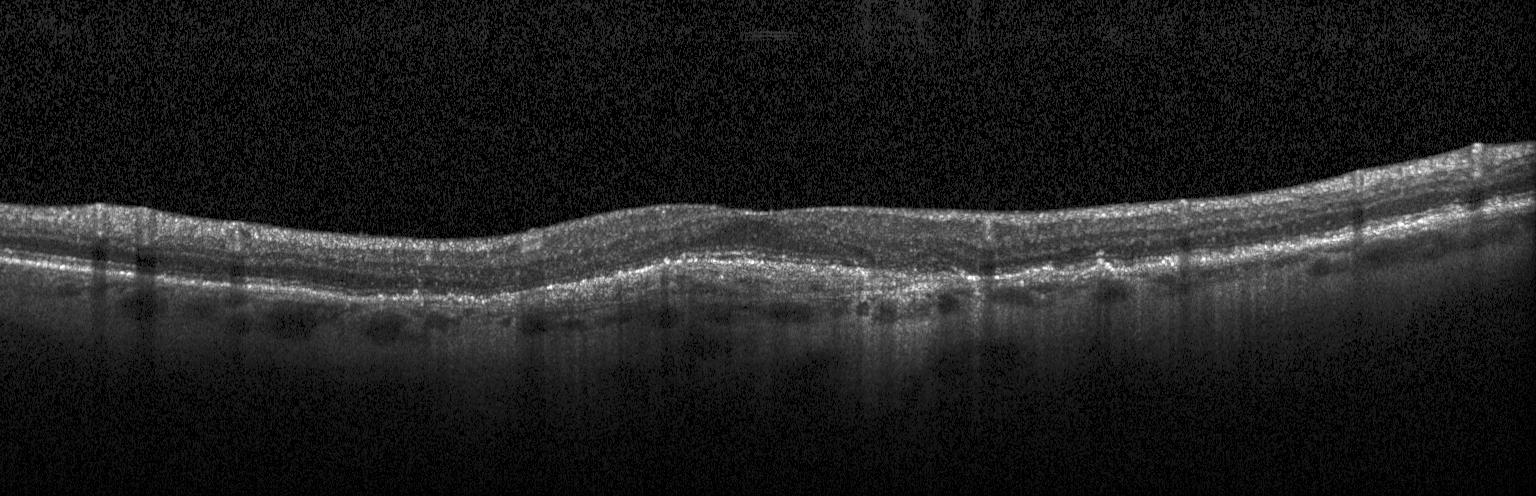 Acquired on a Heidelberg Spectralis; centered on the fovea; OCT line scan; spectral-domain optical coherence tomography
Dx: choroidal neovascularization.